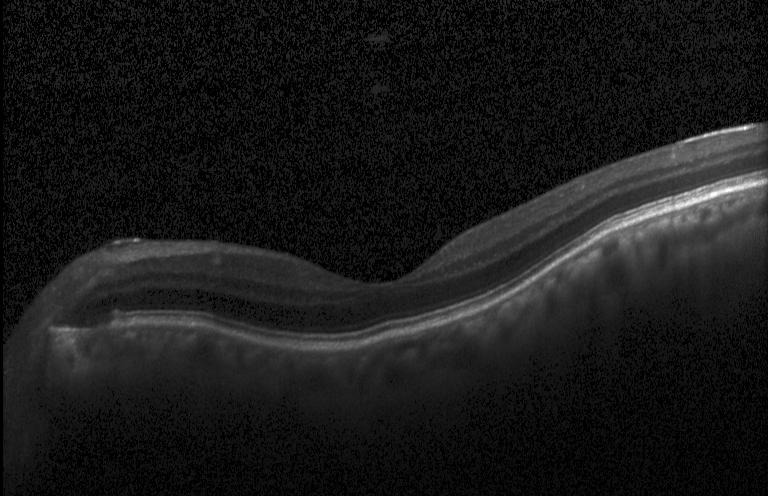

Retinal OCT B-scan; macular scan. OCT finding: no evidence of CNV, DME, or drusen.